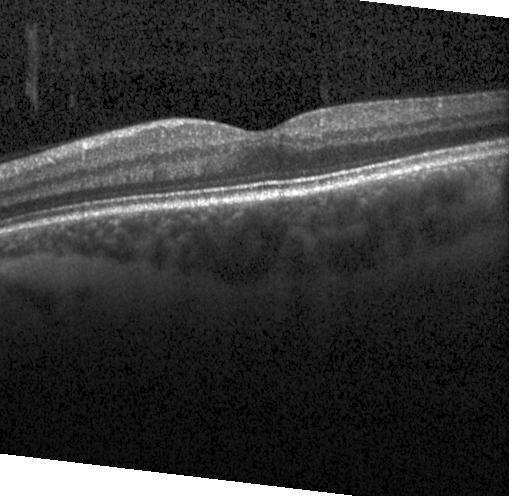 OCT line scan.
Dx: no evidence of choroidal neovascularization, diabetic macular edema, or drusen.